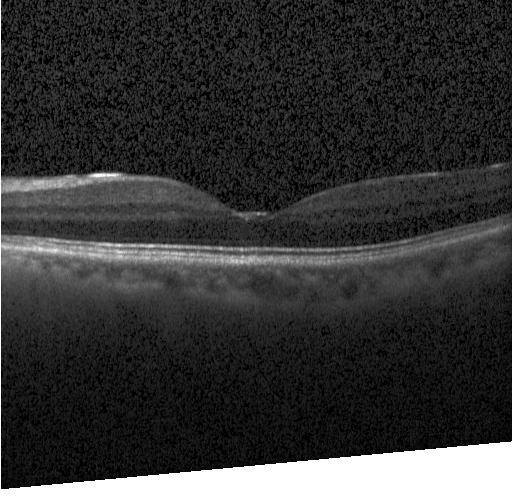

Optical coherence tomography B-scan.
This B-scan demonstrates no choroidal neovascularization, diabetic macular edema, or drusen.